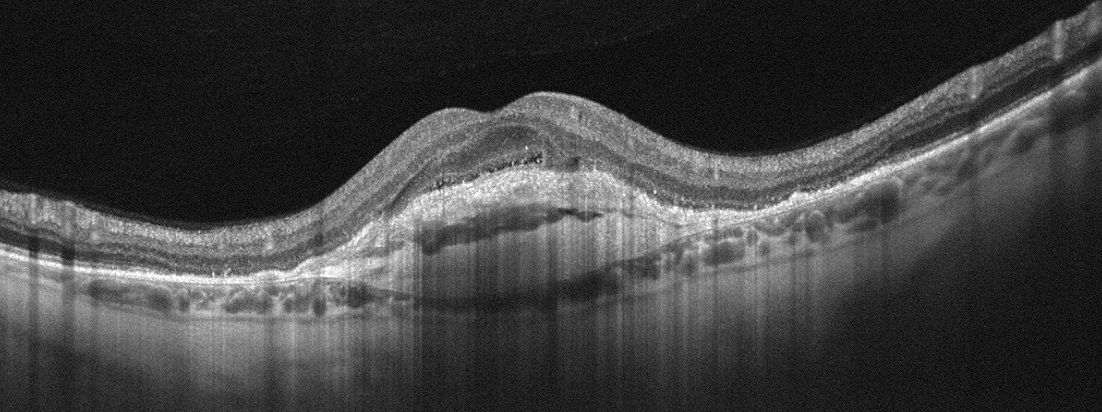

Macular OCT: age-related macular degeneration.